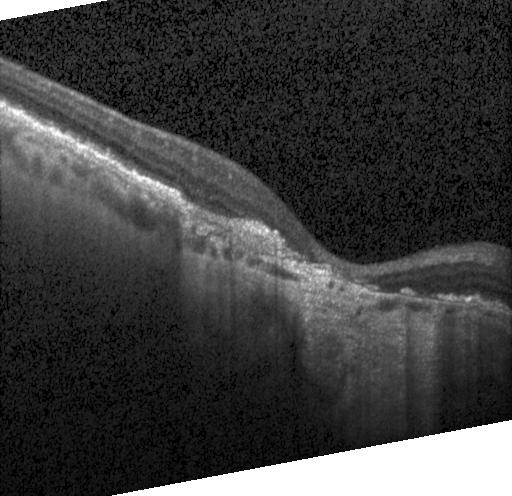

OCT line scan; fovea-centered
Macular OCT: choroidal neovascularization (CNV).